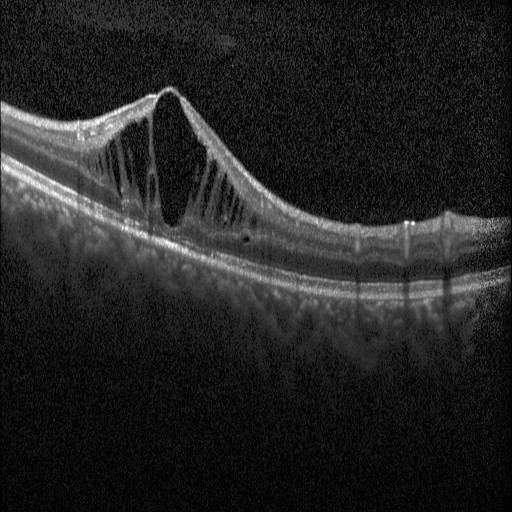
Optical coherence tomography B-scan. Spectral-domain OCT. Centered on the fovea. Heidelberg Spectralis OCT system. Diagnosis: diabetic macular edema.